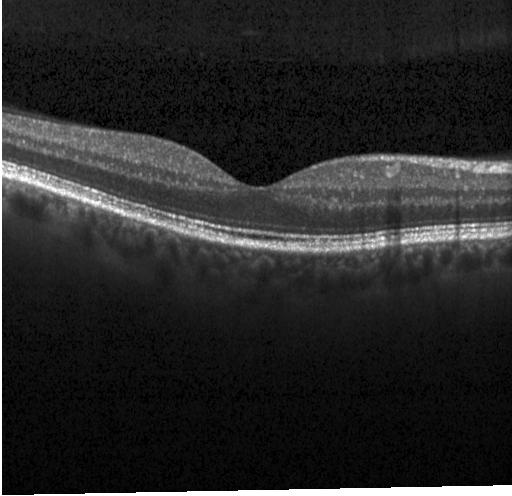 OCT scan showing no evidence of choroidal neovascularization, diabetic macular edema, or drusen.